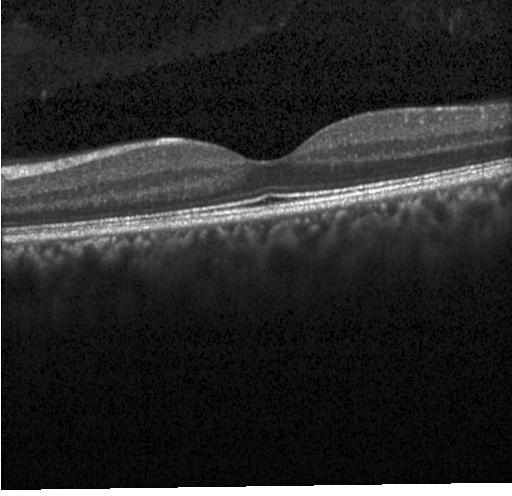
Diagnosis: no evidence of choroidal neovascularization, diabetic macular edema, or drusen.